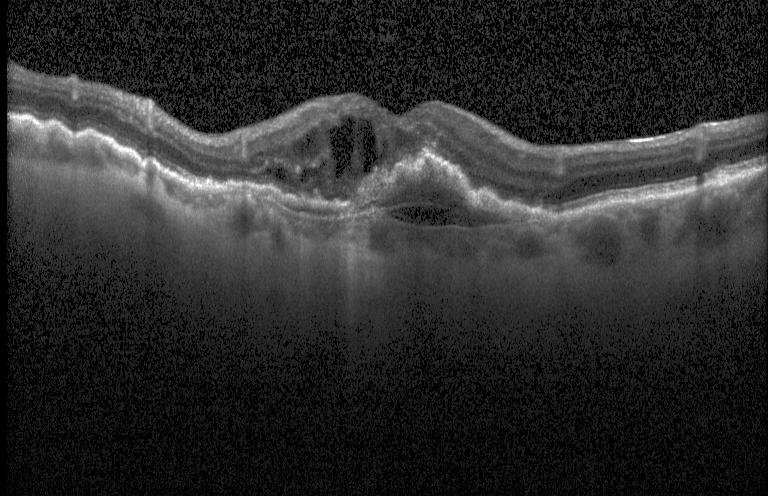
Retinal OCT cross-section.
Diagnosis: a choroidal neovascular membrane.